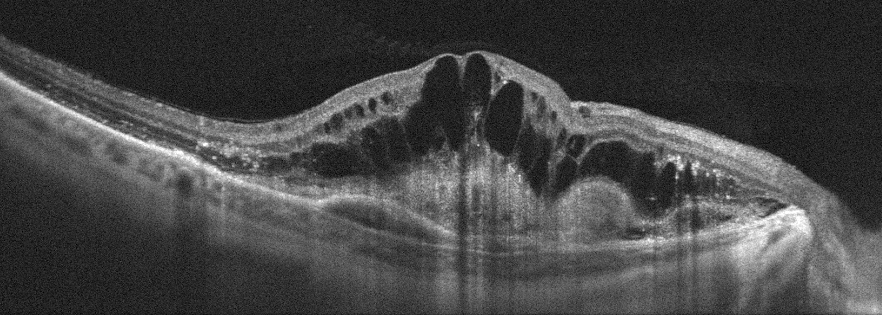
OCT line scan.
Finding: age-related macular degeneration.